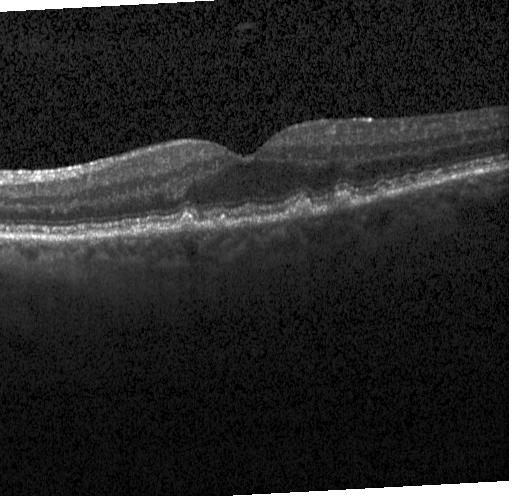

Impression: drusen.